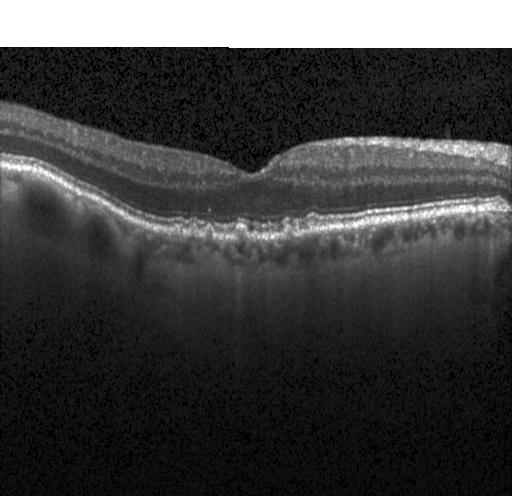
Impression: multiple drusen.